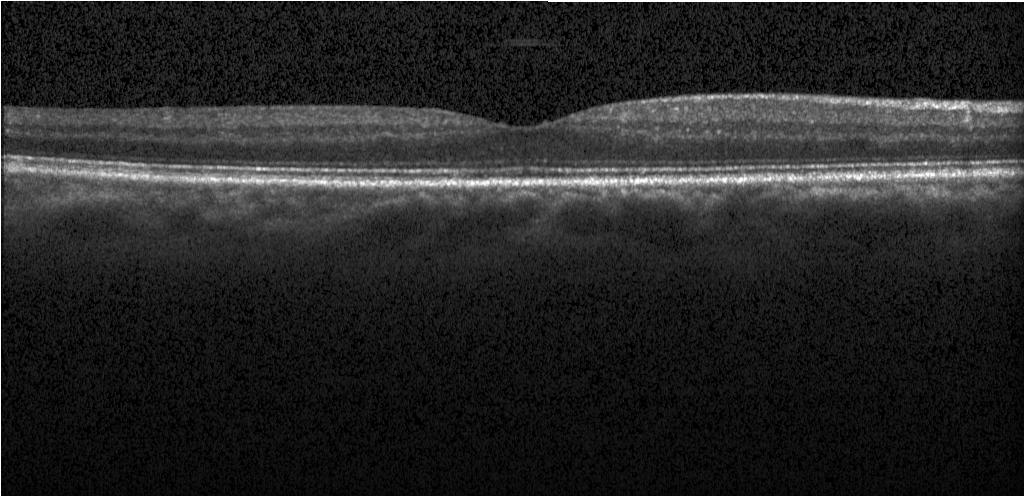
OCT B-scan.
The scan shows no evidence of choroidal neovascularization, diabetic macular edema, or drusen.